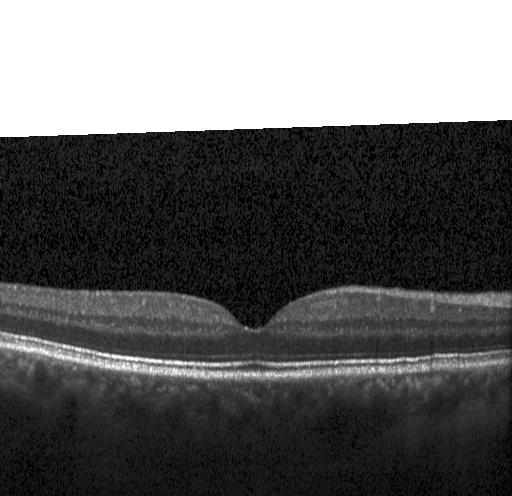
Spectral-domain optical coherence tomography; OCT line scan.
Macular OCT: no CNV, DME, or drusen.